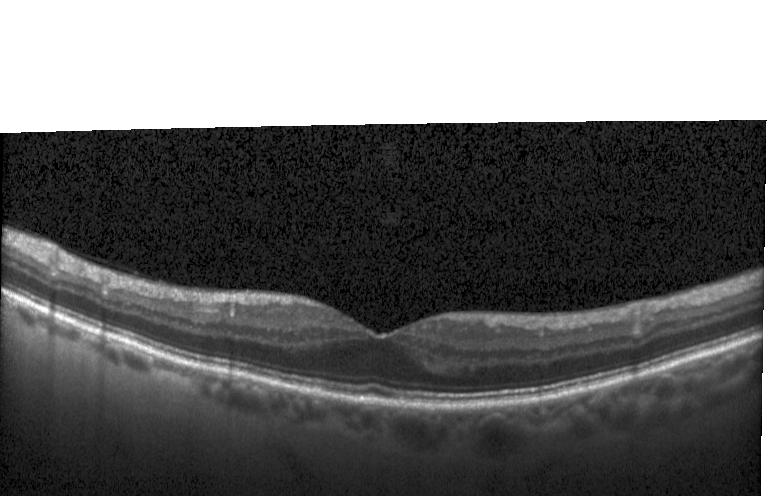
OCT B-scan; spectral-domain OCT.
Diagnosis: neither CNV, DME, nor drusen.